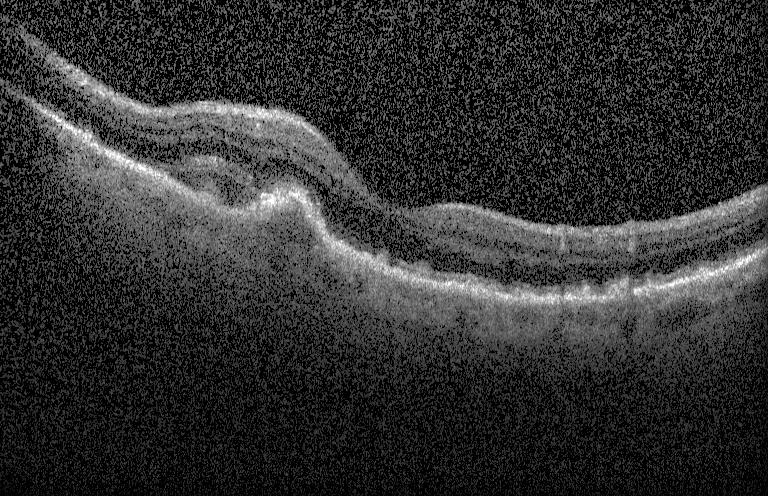 Spectral-domain OCT B-scan: a choroidal neovascular membrane.